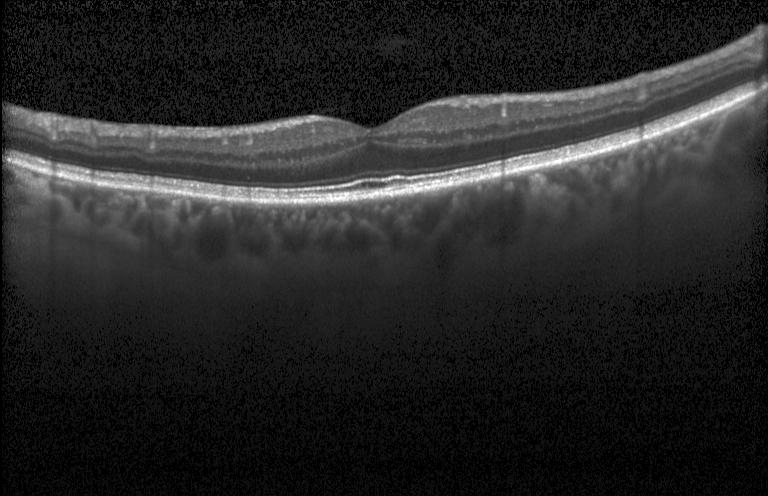
Retinal OCT cross-section showing no evidence of choroidal neovascularization, diabetic macular edema, or drusen.